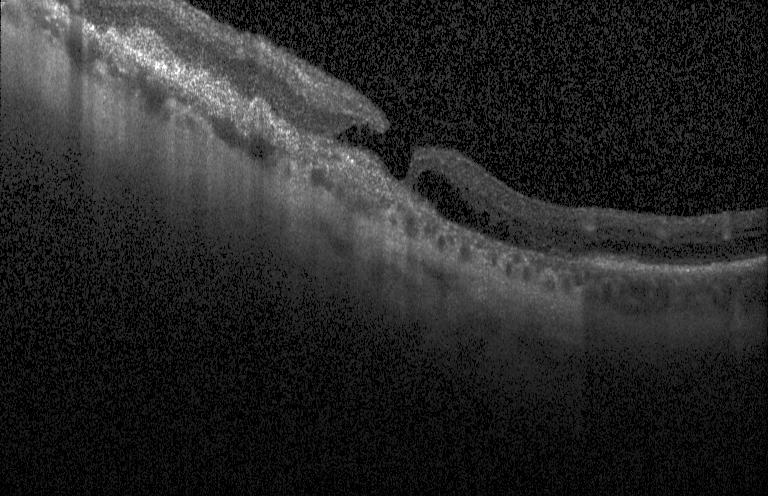
Retinal OCT B-scan · spectral-domain optical coherence tomography.
The scan shows a choroidal neovascular membrane.